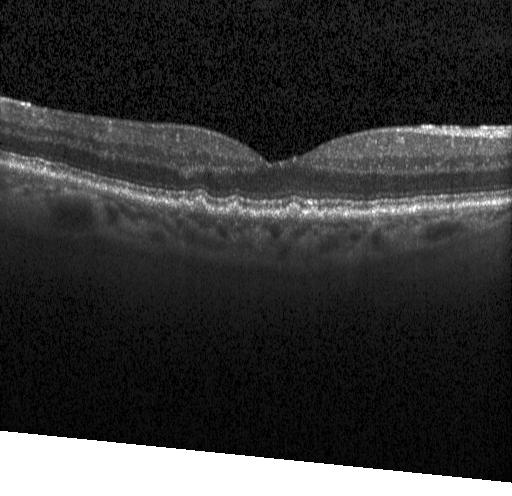 Impression: drusen.